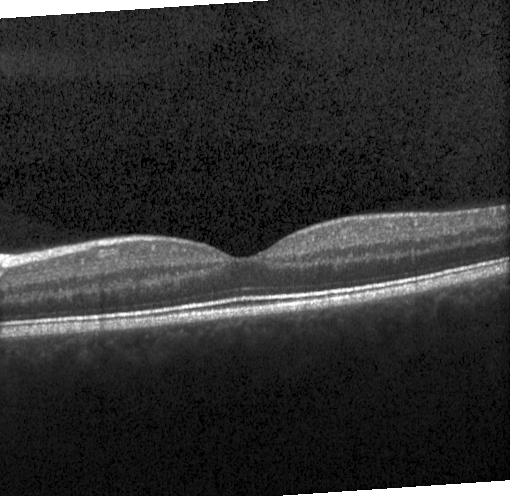 OCT line scan. Finding: neither choroidal neovascularization, diabetic macular edema, nor drusen.